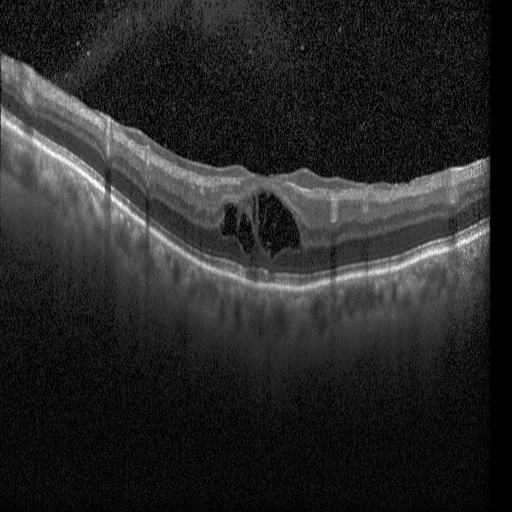

OCT B-scan, acquired on a Heidelberg Spectralis, SD-OCT, horizontal scan through the fovea
Finding: diabetic macular edema.